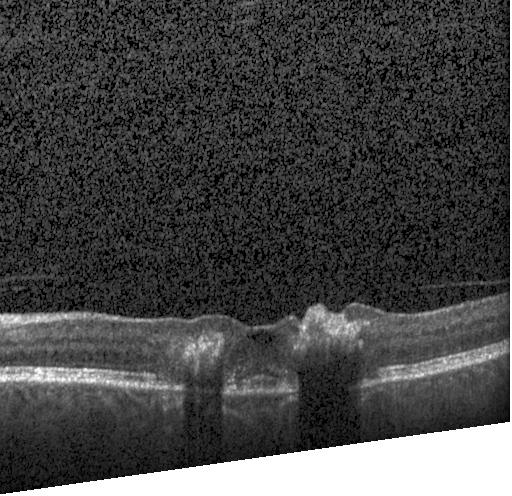 Spectral-domain OCT B-scan: a choroidal neovascular membrane.